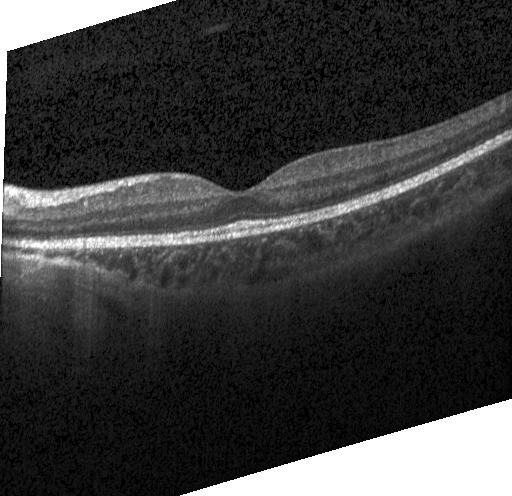

Acquired on a Heidelberg Spectralis · horizontal scan through the fovea · OCT B-scan · spectral-domain optical coherence tomography. Diagnosis: no CNV, DME, or drusen.